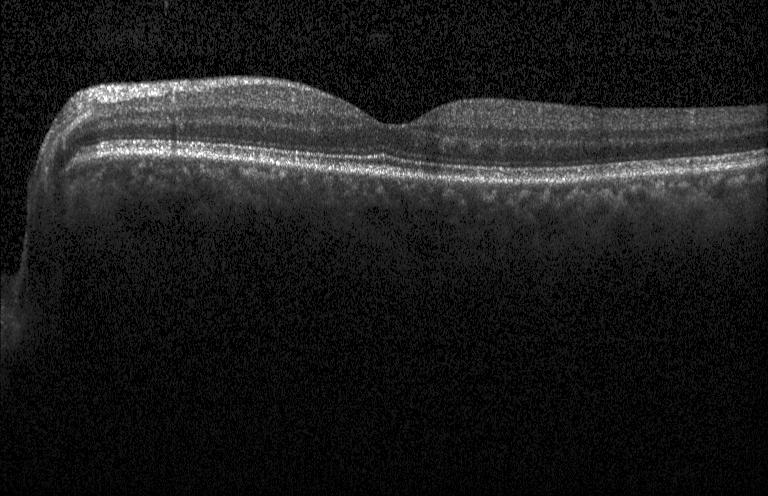 Retinal OCT B-scan · spectral-domain OCT · Heidelberg Spectralis OCT system. No choroidal neovascularization, diabetic macular edema, or drusen.